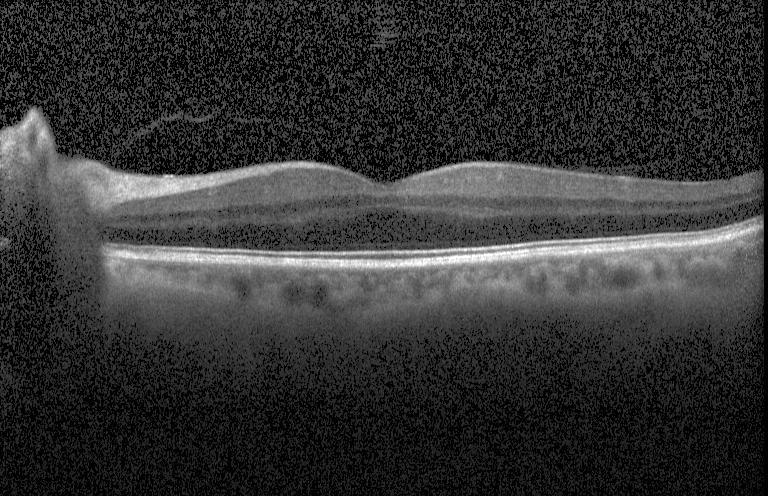 Impression: neither choroidal neovascularization, diabetic macular edema, nor drusen.